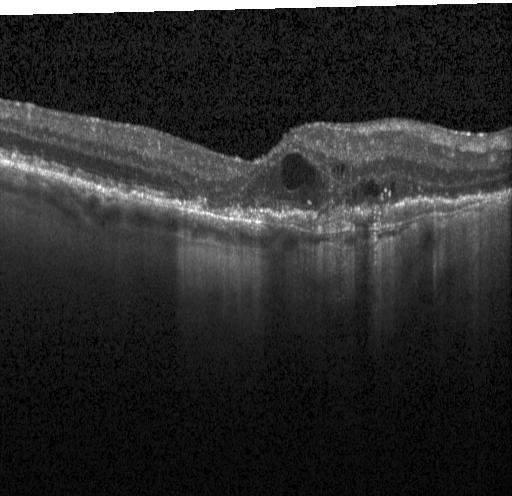
Impression: choroidal neovascularization (CNV).